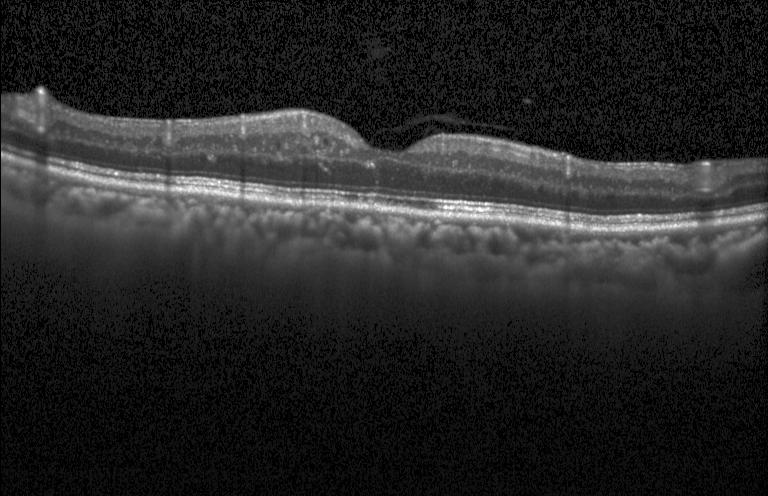 Impression: no evidence of choroidal neovascularization, diabetic macular edema, or drusen.